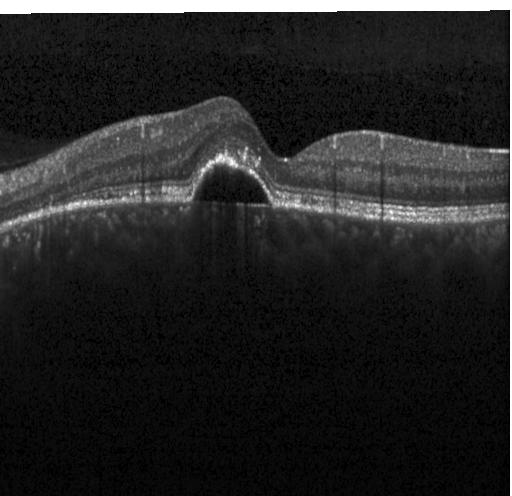

Optical coherence tomography scan
Finding: a choroidal neovascular membrane.